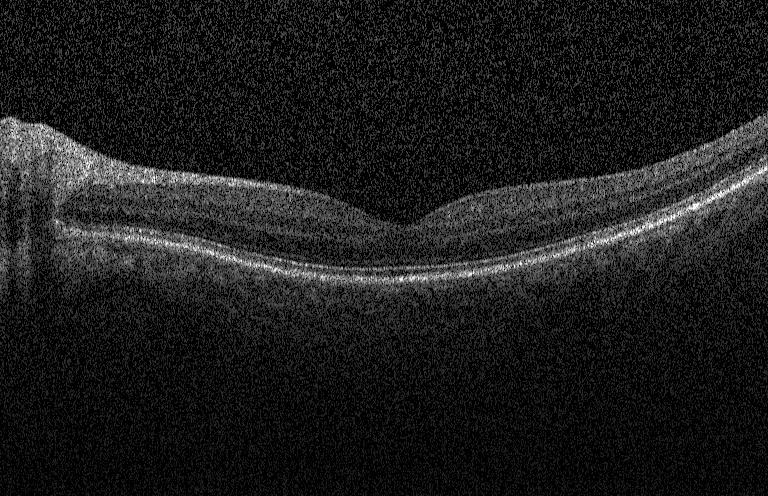 Horizontal scan through the fovea, instrument: Heidelberg Spectralis, spectral-domain optical coherence tomography, retinal OCT cross-section
Impression: no choroidal neovascularization, diabetic macular edema, or drusen.